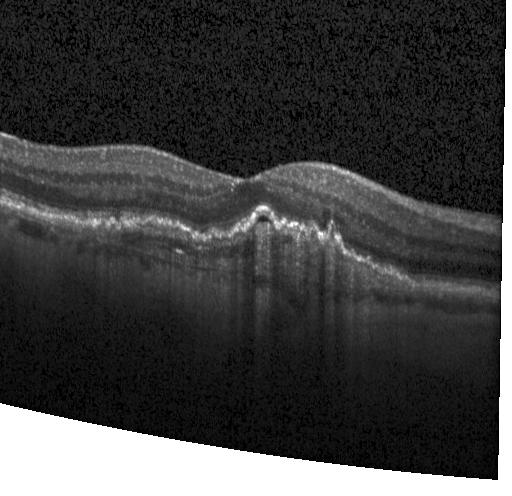 OCT line scan. Heidelberg Spectralis. Spectral-domain optical coherence tomography. Through the macula. Diagnosis: a choroidal neovascular membrane.